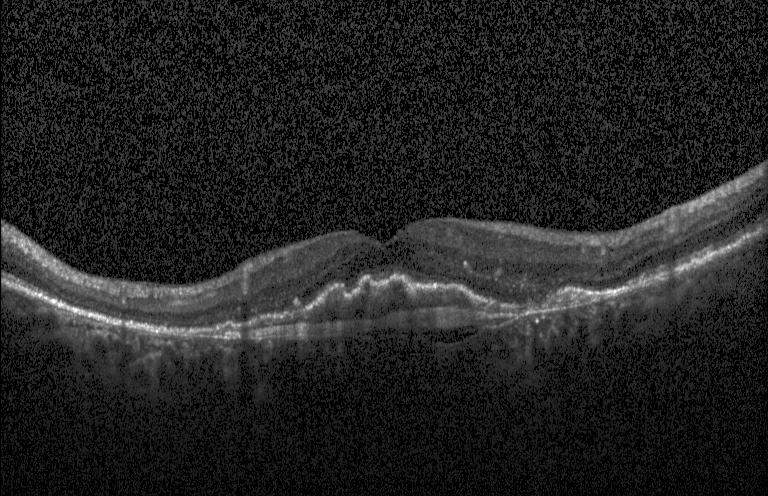 Retinal OCT B-scan; spectral-domain optical coherence tomography; macular scan.
Assessment: choroidal neovascularization.